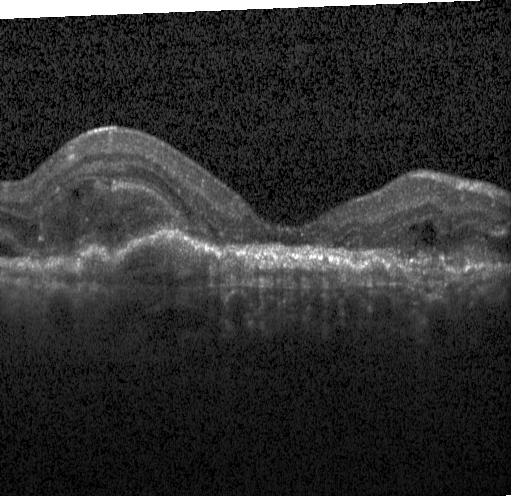 OCT scan showing choroidal neovascularization (CNV).